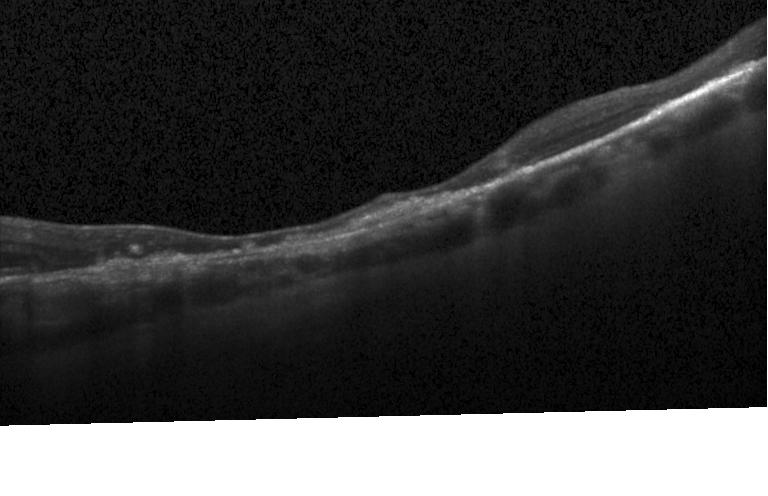
Retinal OCT cross-section.
The scan shows CNV.